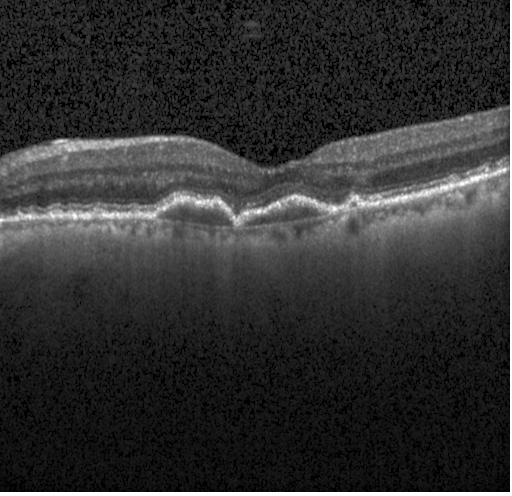 SD-OCT. OCT line scan. OCT finding: choroidal neovascularization (CNV).